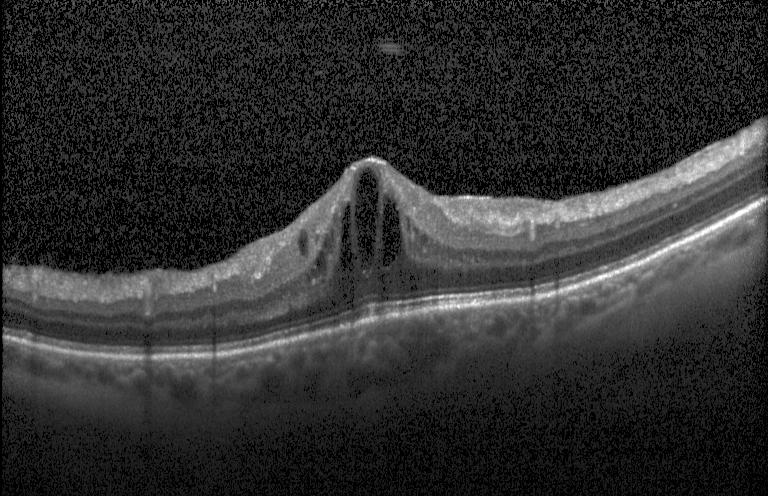

Spectral-domain OCT; OCT line scan — Assessment: diabetic macular edema (DME).